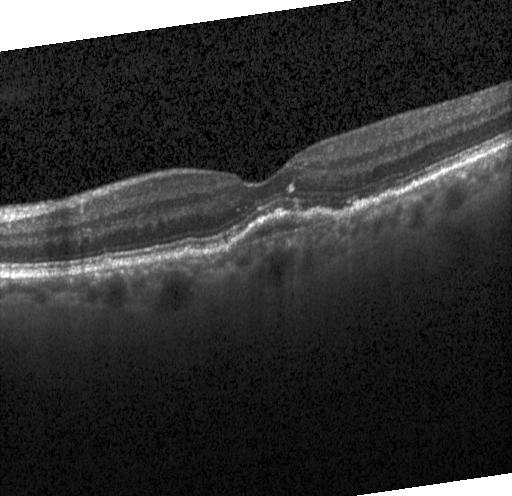
Retinal OCT B-scan
Finding: a choroidal neovascular membrane.